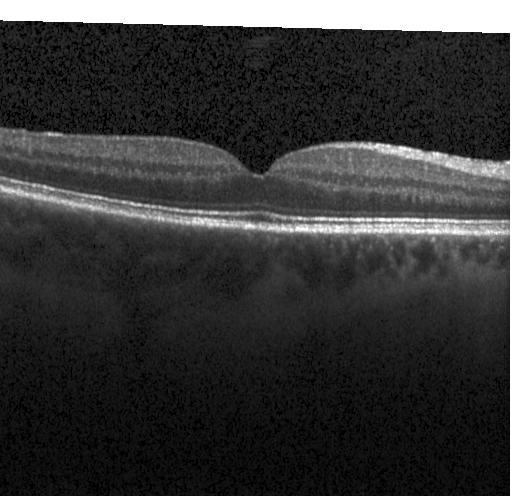
OCT finding: no evidence of choroidal neovascularization, diabetic macular edema, or drusen.